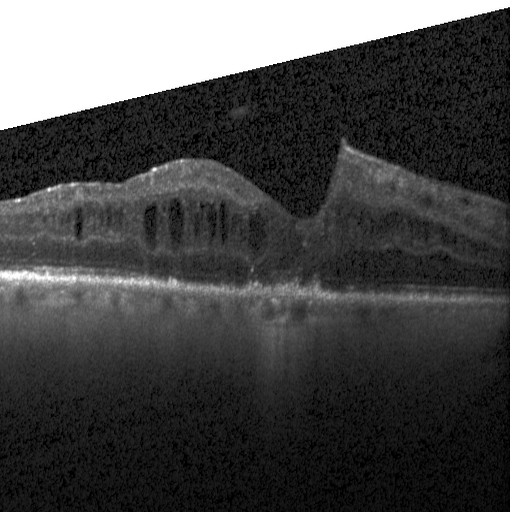 Acquired on a Heidelberg Spectralis, centered on the fovea, retinal OCT cross-section. OCT finding: diabetic macular edema (DME).